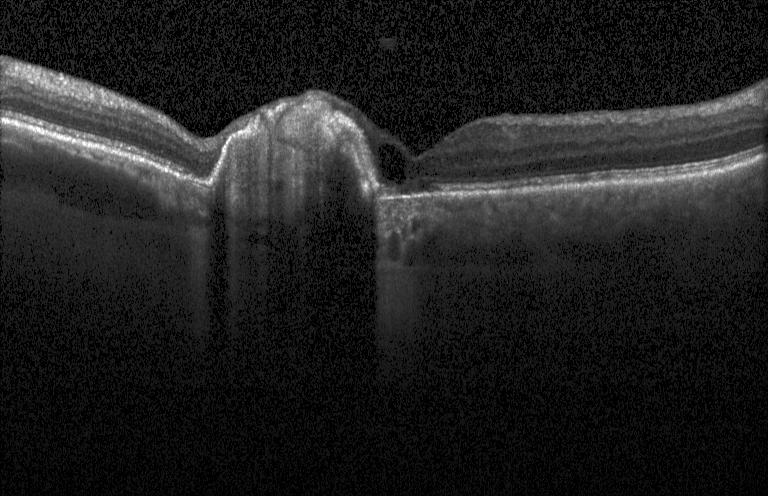 Retinal OCT cross-section
This B-scan demonstrates a choroidal neovascular membrane.